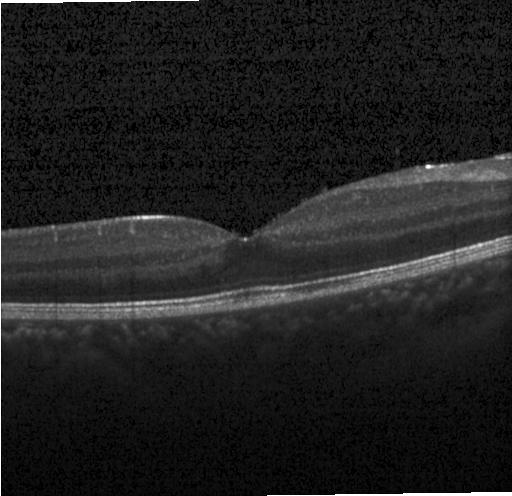

Heidelberg Spectralis · retinal OCT cross-section · fovea-centered · spectral-domain optical coherence tomography.
OCT finding: no CNV, no DME, and no drusen.